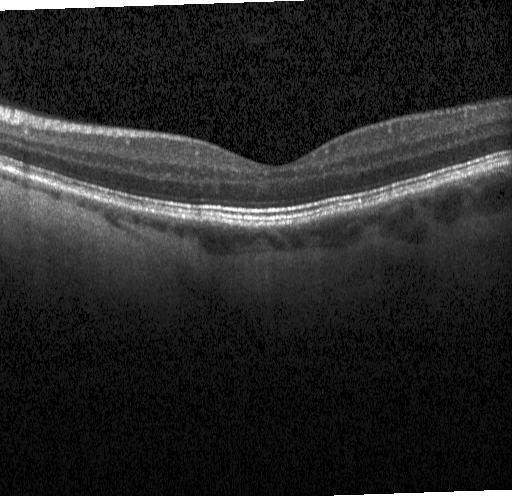 OCT B-scan. Diagnosis: no choroidal neovascularization, no diabetic macular edema, and no drusen.